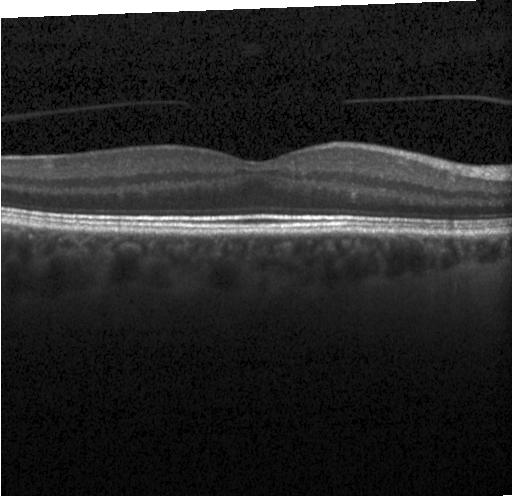 Macular OCT: no CNV, DME, or drusen.